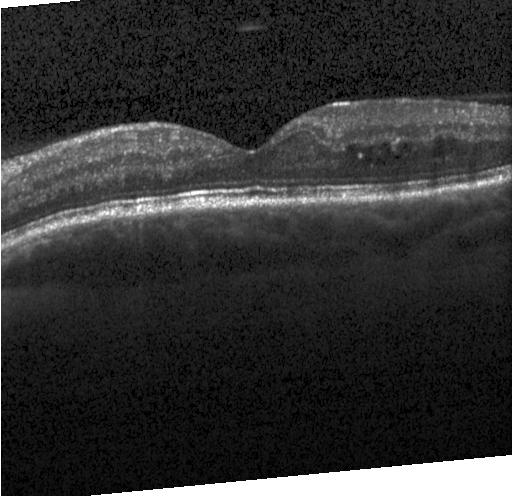 Optical coherence tomography scan
This B-scan demonstrates diabetic macular edema (DME).